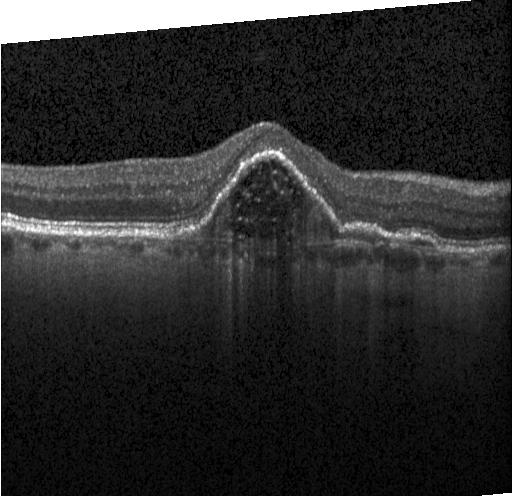

Retinal OCT cross-section · horizontal scan through the fovea · Heidelberg Spectralis · SD-OCT — Impression: CNV.